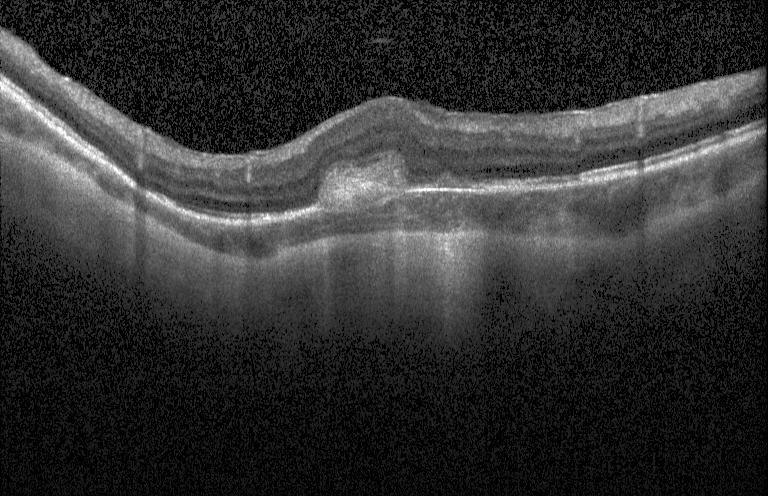

Acquired on a Heidelberg Spectralis, optical coherence tomography B-scan. A choroidal neovascular membrane.